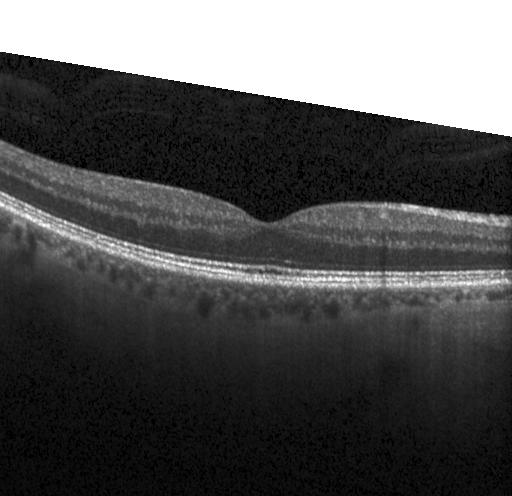 Diagnosis: no choroidal neovascularization, diabetic macular edema, or drusen.